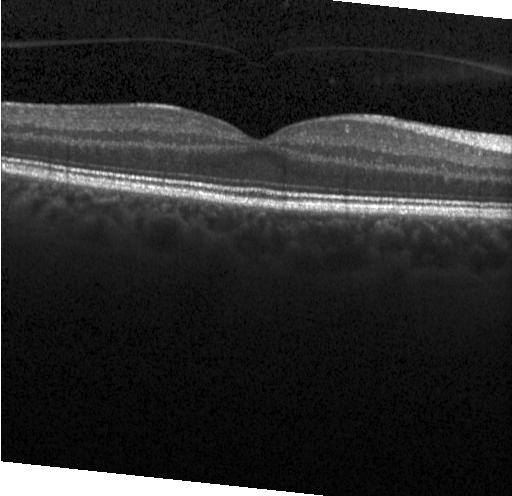

Retinal OCT cross-section, fovea-centered, spectral-domain OCT.
Impression: no evidence of CNV, DME, or drusen.